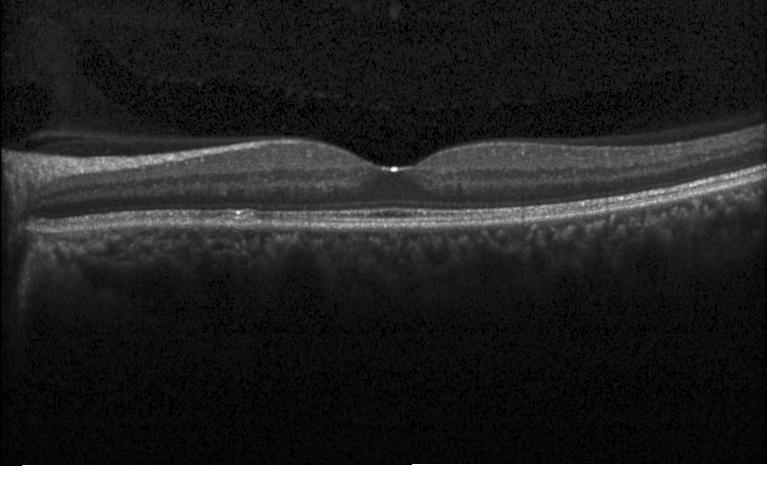 Macular scan; spectral-domain OCT; retinal OCT B-scan; Heidelberg Spectralis
Finding: neither CNV, DME, nor drusen.